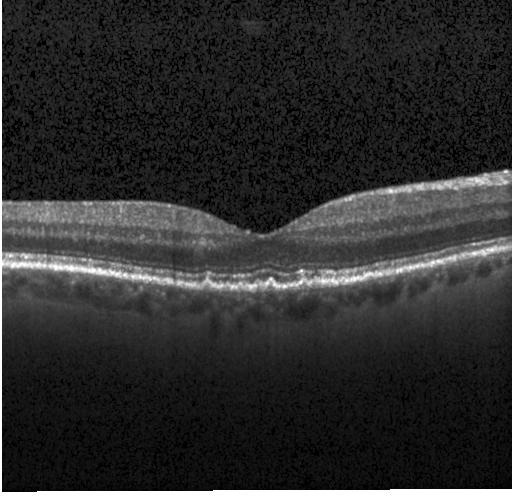

Fovea-centered; optical coherence tomography B-scan — This B-scan demonstrates sub-RPE drusenoid deposits.